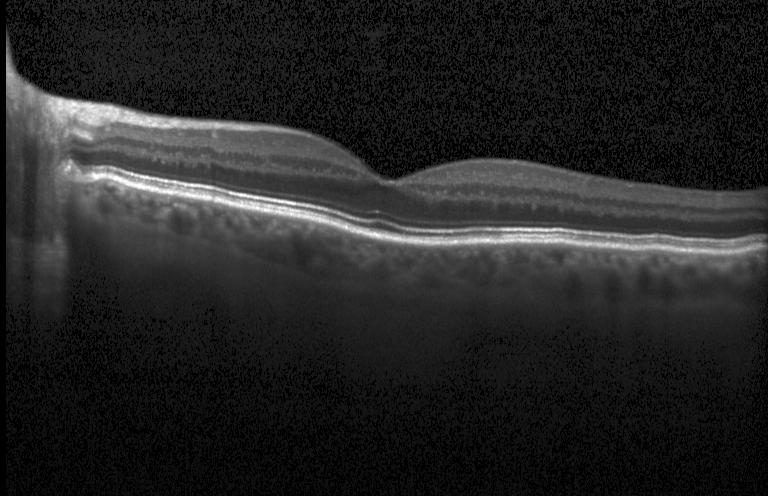 Horizontal scan through the fovea, OCT line scan, spectral-domain OCT. Impression: no evidence of choroidal neovascularization, diabetic macular edema, or drusen.